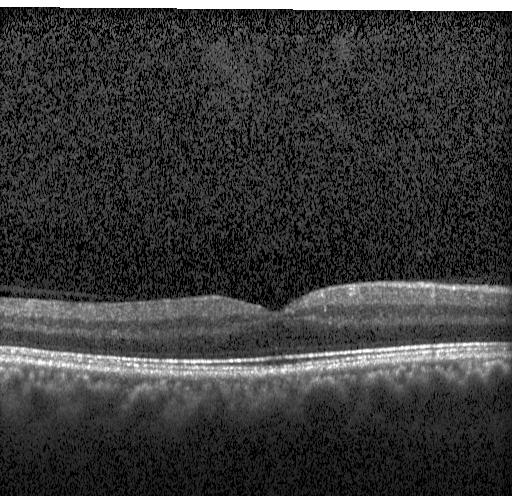

Optical coherence tomography B-scan; through the macula; Heidelberg Spectralis; spectral-domain OCT — Diagnosis: no choroidal neovascularization, diabetic macular edema, or drusen.